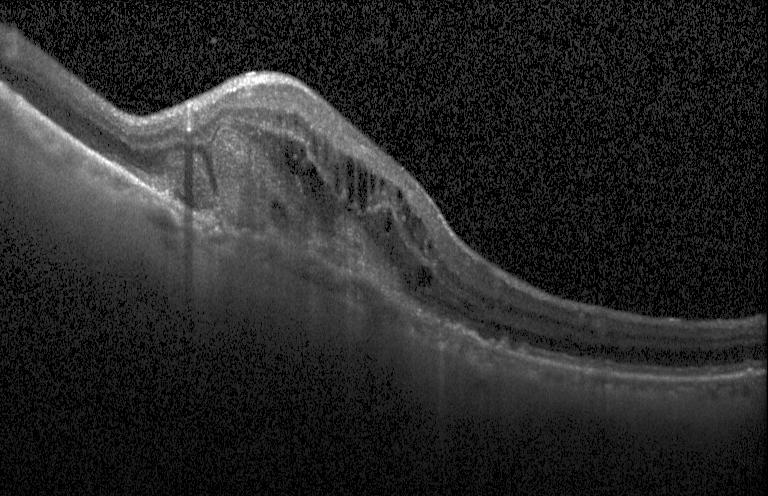

Macular OCT demonstrating CNV.